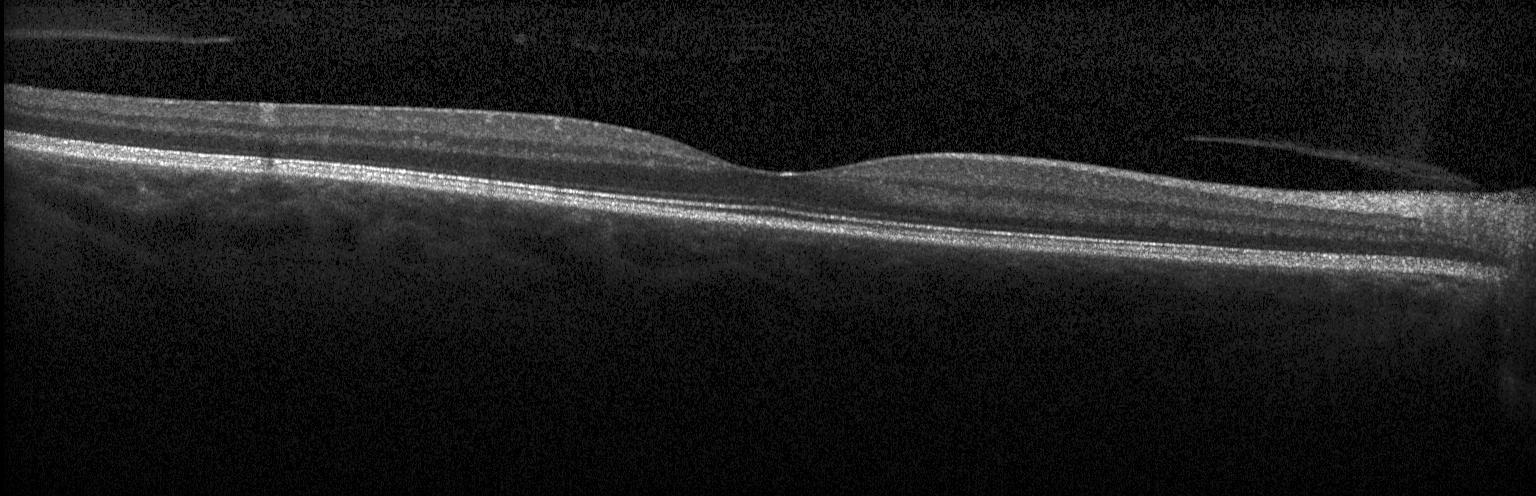 Neither choroidal neovascularization, diabetic macular edema, nor drusen.